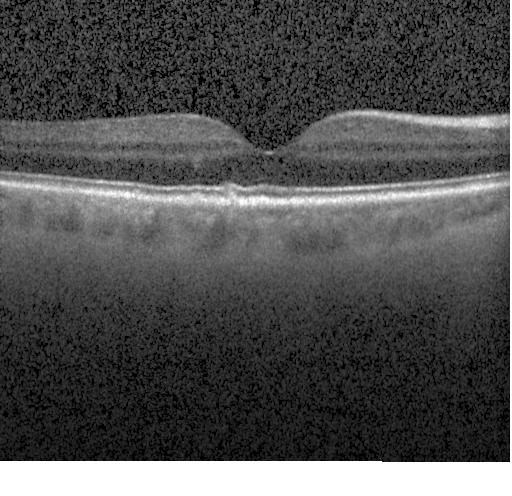

OCT finding: sub-RPE drusenoid deposits.